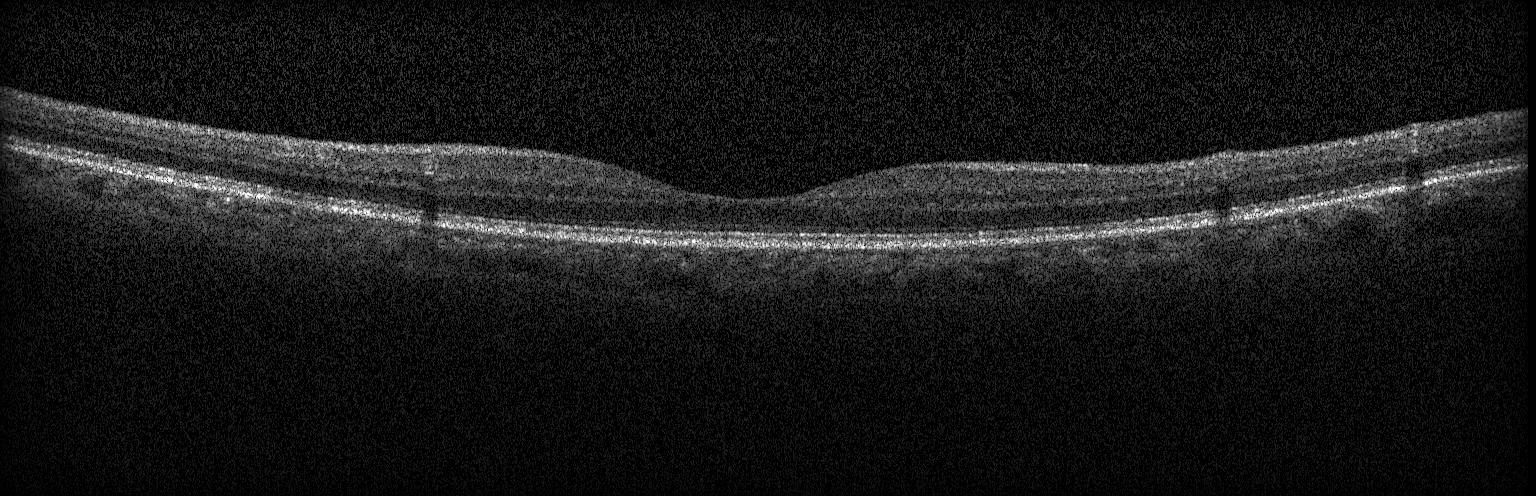
Macular OCT demonstrating no evidence of choroidal neovascularization, diabetic macular edema, or drusen.